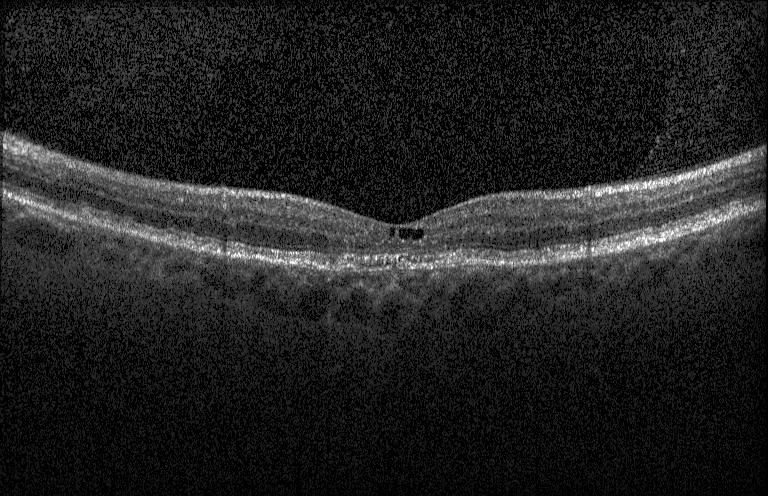 Finding: a choroidal neovascular membrane.